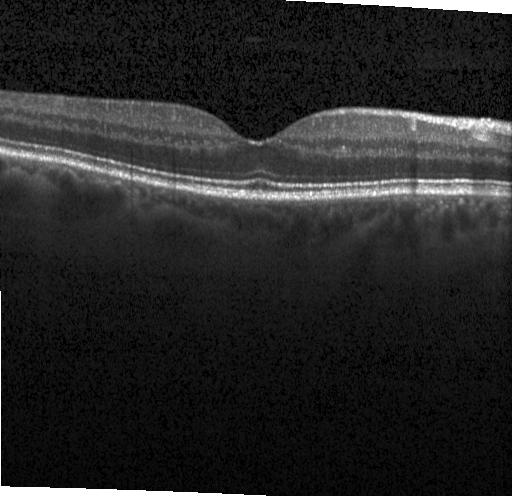

Dx: neither CNV, DME, nor drusen.